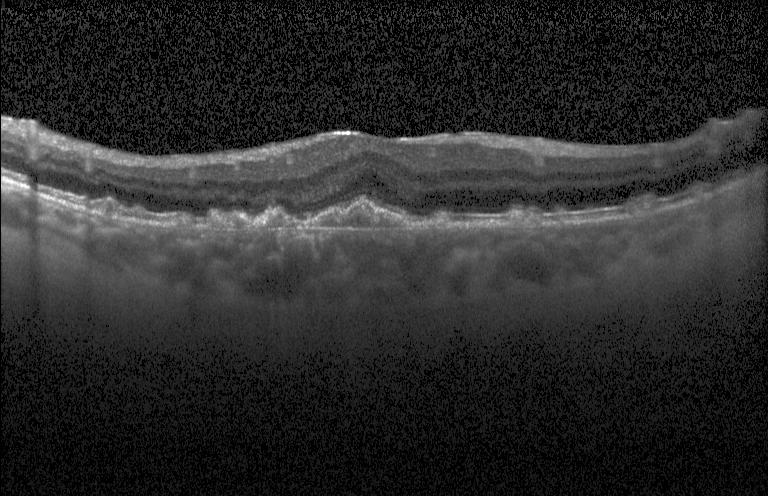

A choroidal neovascular membrane.